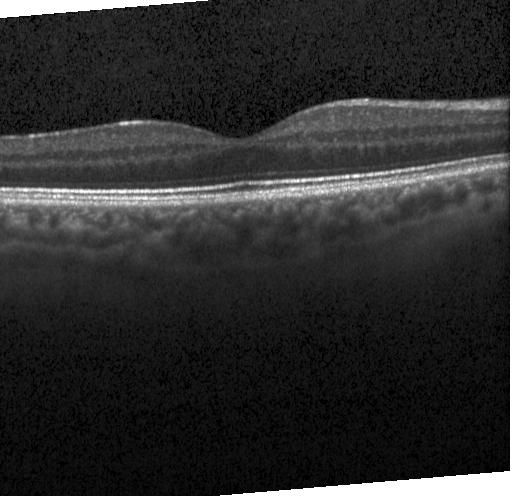
OCT B-scan
This B-scan demonstrates neither choroidal neovascularization, diabetic macular edema, nor drusen.